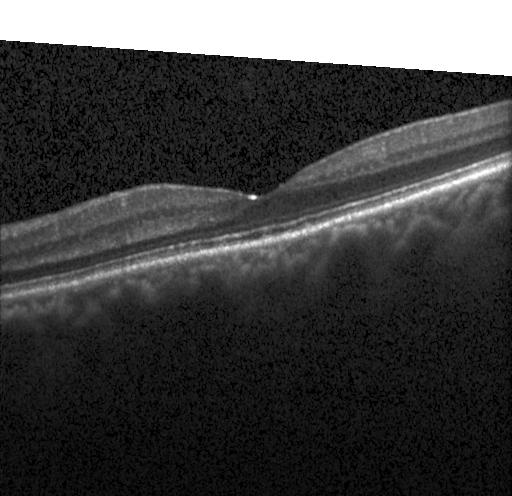 Heidelberg Spectralis. SD-OCT. Fovea-centered. Retinal OCT B-scan — Impression: no evidence of choroidal neovascularization, diabetic macular edema, or drusen.